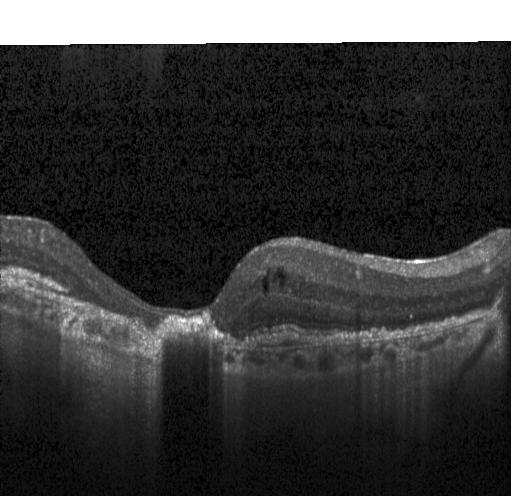

OCT line scan. Centered on the fovea. Heidelberg Spectralis OCT system. SD-OCT. A choroidal neovascular membrane.